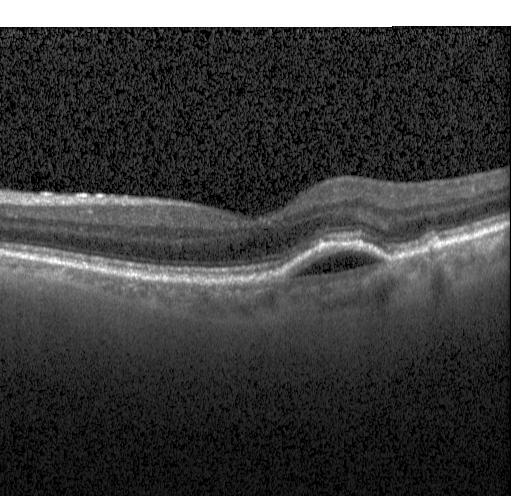
Spectral-domain optical coherence tomography. Retinal OCT B-scan
OCT finding: a choroidal neovascular membrane.